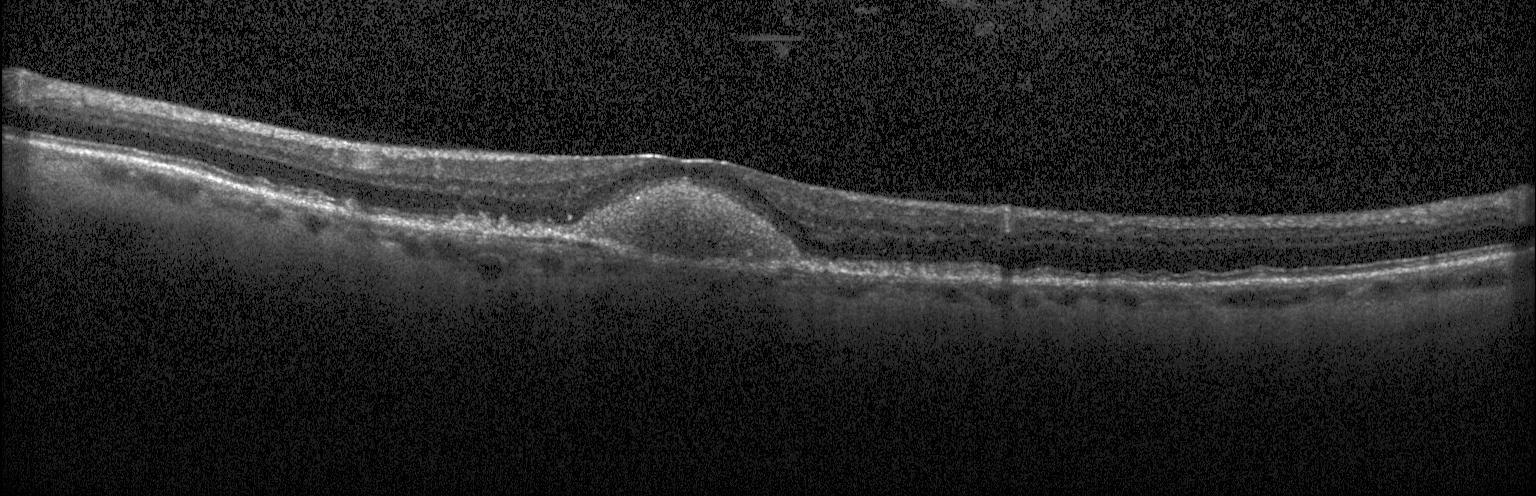
SD-OCT, retinal OCT B-scan, acquired on a Heidelberg Spectralis. Assessment: CNV.